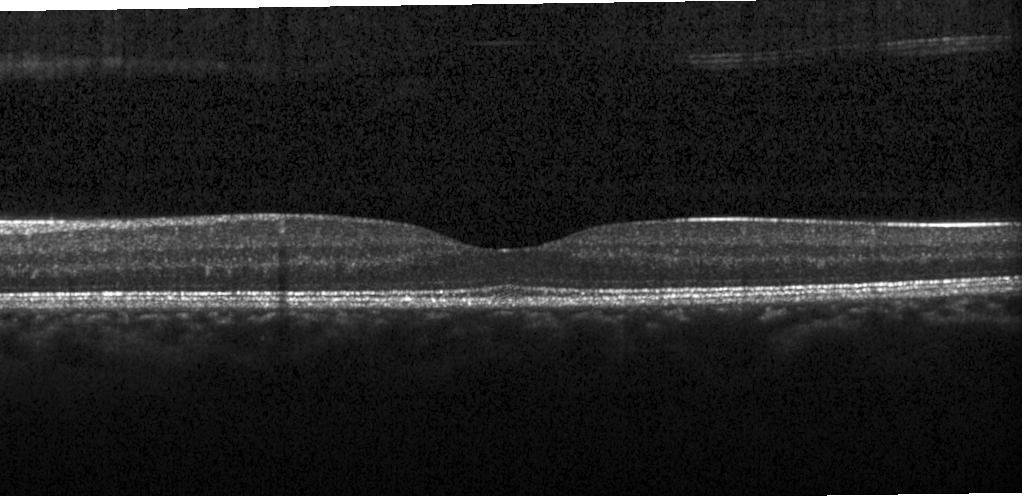
Retinal OCT B-scan. The scan shows no choroidal neovascularization, no diabetic macular edema, and no drusen.